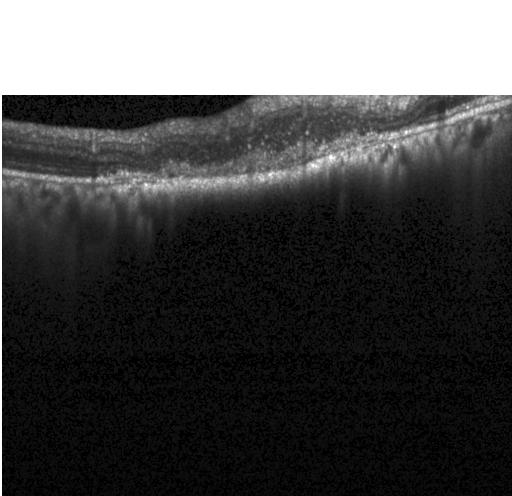

Retinal OCT cross-section. A choroidal neovascular membrane.